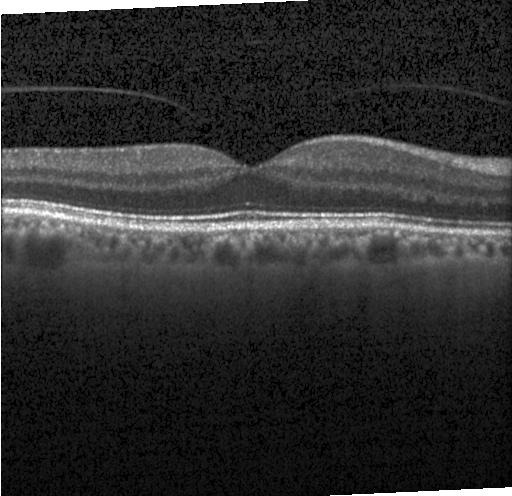

OCT scan showing neither CNV, DME, nor drusen.